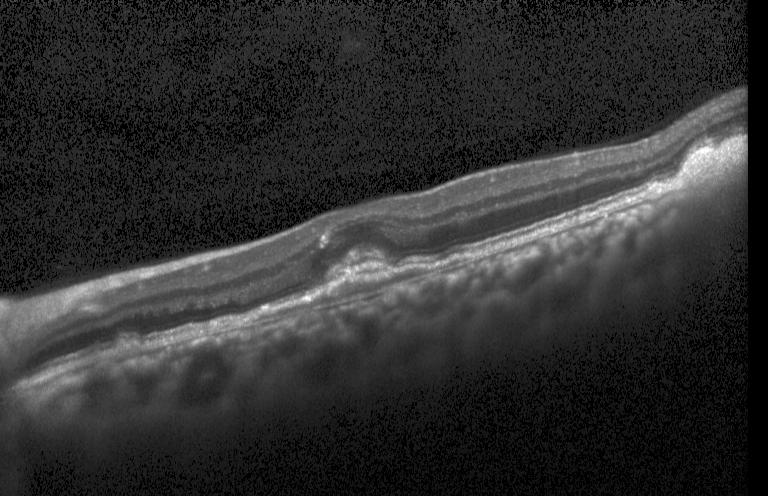

OCT scan showing choroidal neovascularization (CNV).